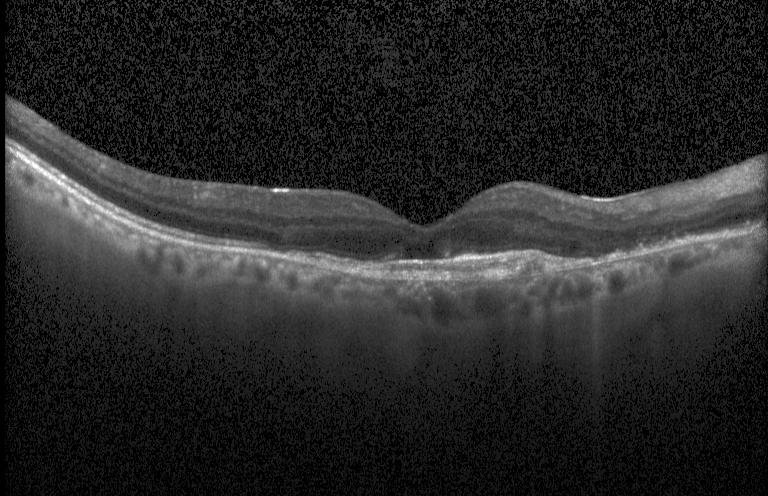 OCT B-scan
Assessment: a choroidal neovascular membrane.